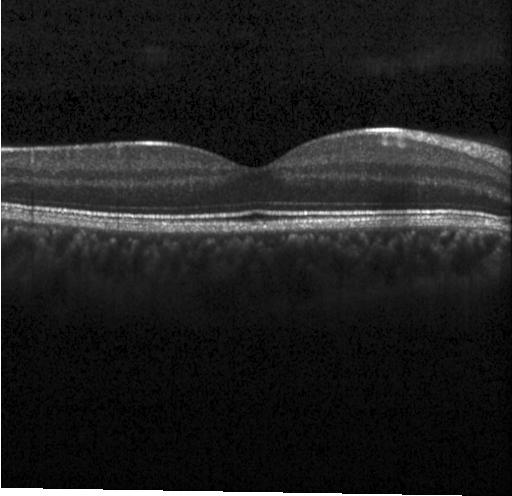
Instrument: Heidelberg Spectralis · retinal OCT cross-section. This B-scan demonstrates no evidence of choroidal neovascularization, diabetic macular edema, or drusen.